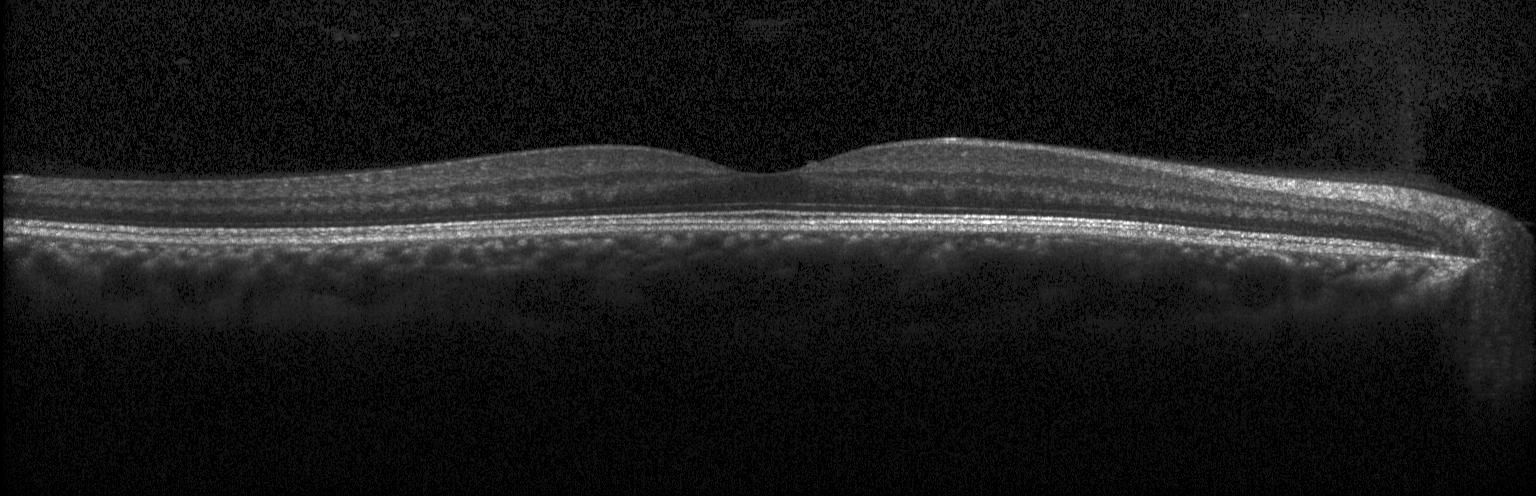
Spectral-domain optical coherence tomography, retinal OCT B-scan. This B-scan demonstrates no evidence of choroidal neovascularization, diabetic macular edema, or drusen.